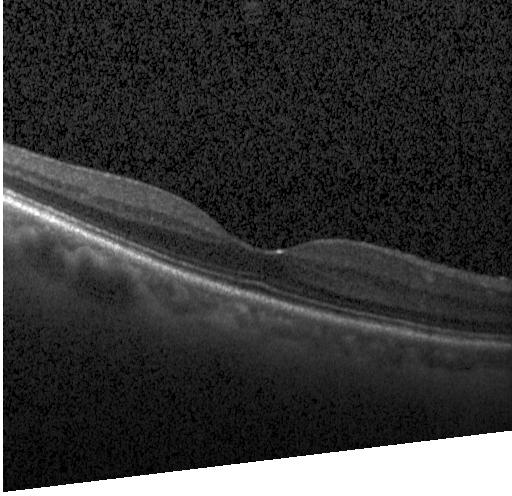
Spectral-domain optical coherence tomography; through the macula; retinal OCT cross-section — Impression: neither CNV, DME, nor drusen.